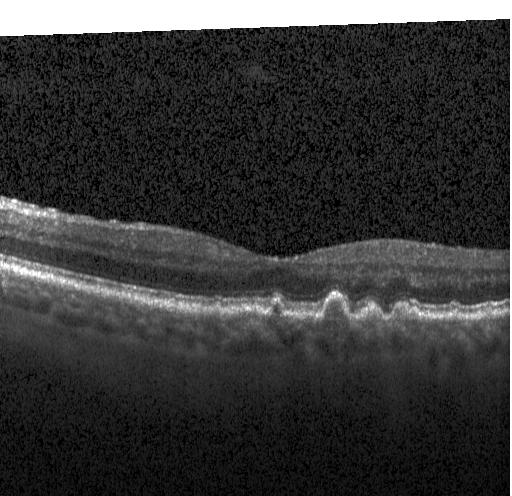 OCT B-scan · through the macula.
OCT finding: drusen.